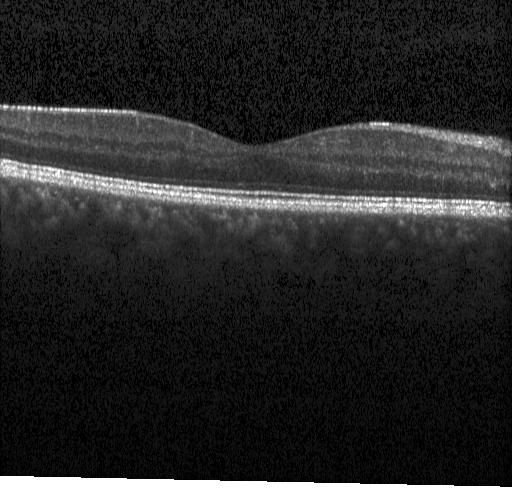

Finding: no evidence of CNV, DME, or drusen.